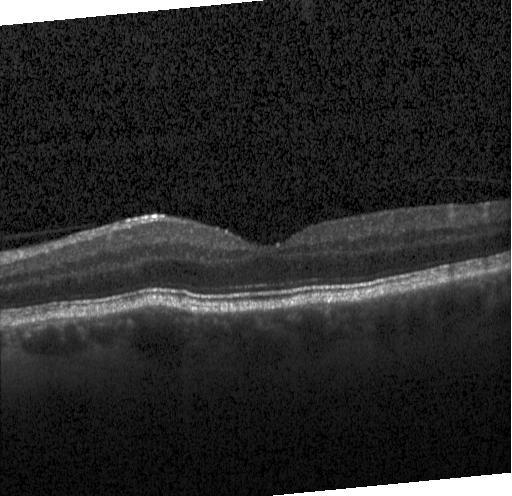

Finding: no evidence of choroidal neovascularization, diabetic macular edema, or drusen.